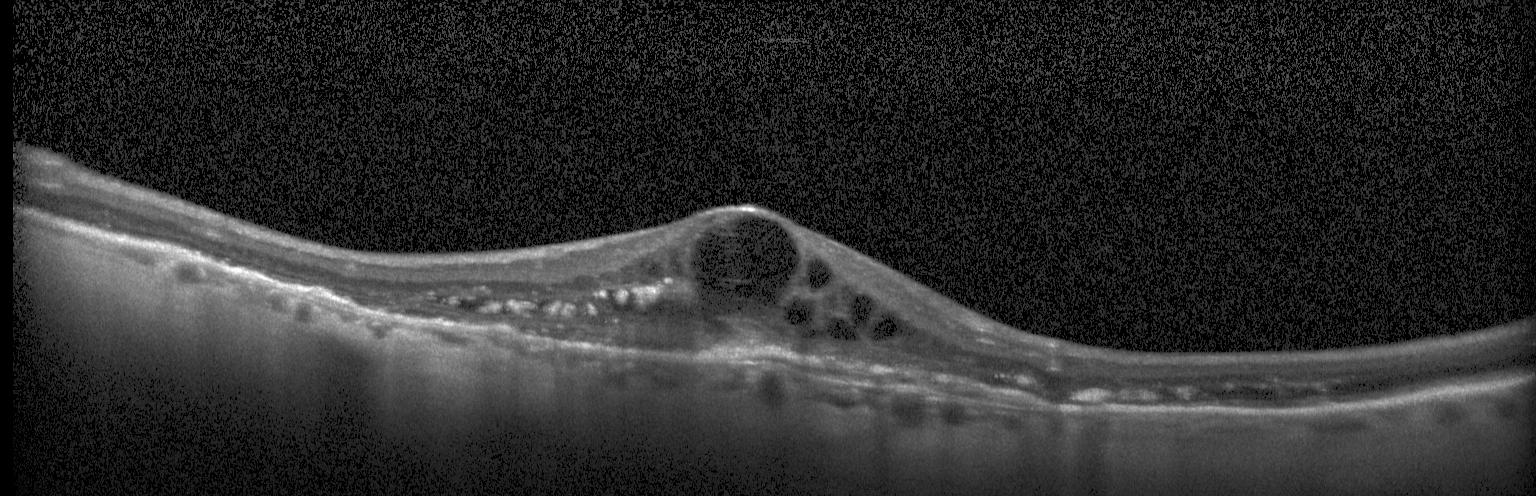
Acquired on a Heidelberg Spectralis, spectral-domain OCT, through the macula, OCT B-scan. Assessment: a choroidal neovascular membrane.